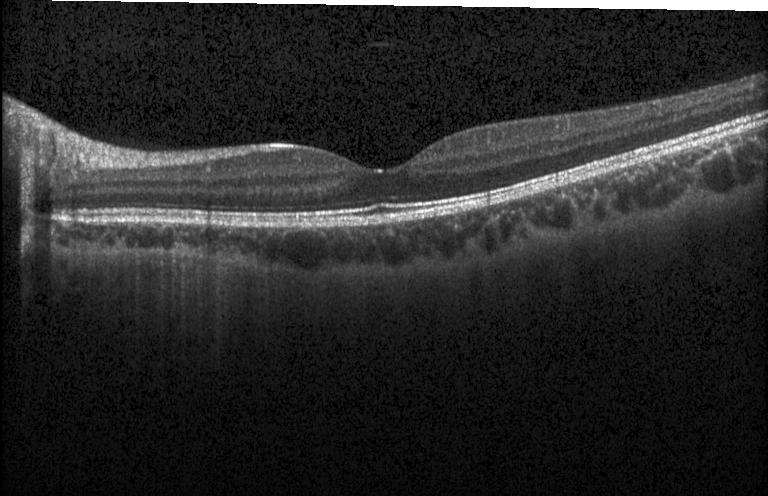 Finding: no evidence of choroidal neovascularization, diabetic macular edema, or drusen.